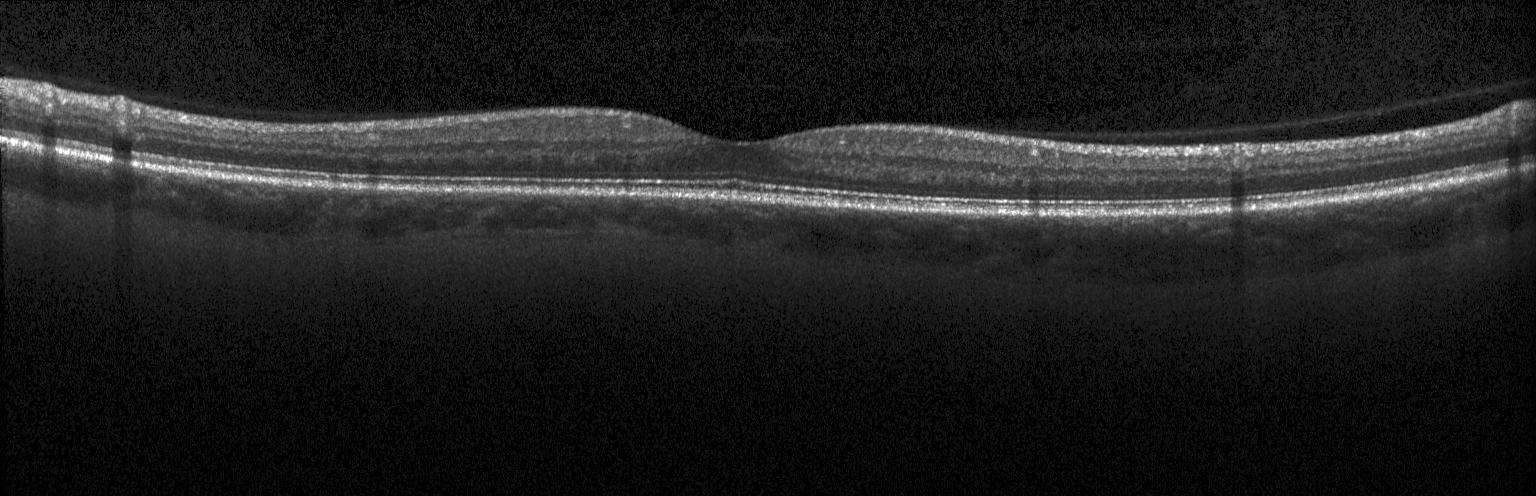

Spectral-domain OCT, OCT B-scan, acquired on a Heidelberg Spectralis, horizontal scan through the fovea
Finding: neither CNV, DME, nor drusen.